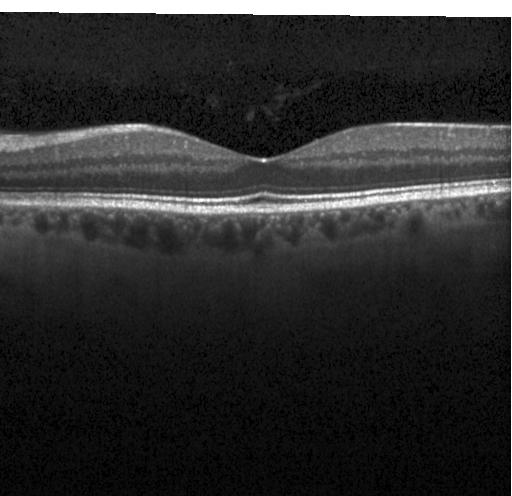

Retinal OCT cross-section, SD-OCT, fovea-centered. Diagnosis: neither choroidal neovascularization, diabetic macular edema, nor drusen.